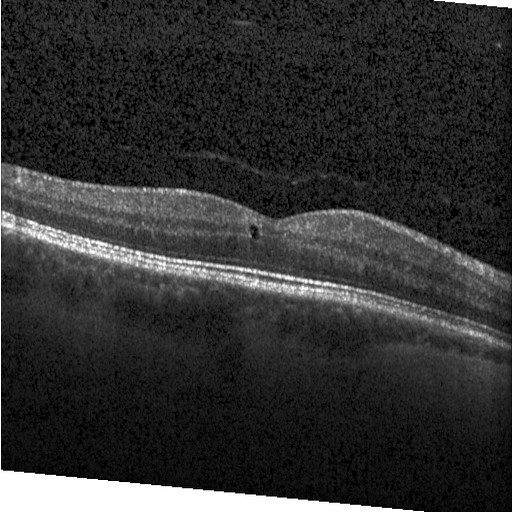
Finding: diabetic macular edema (DME).